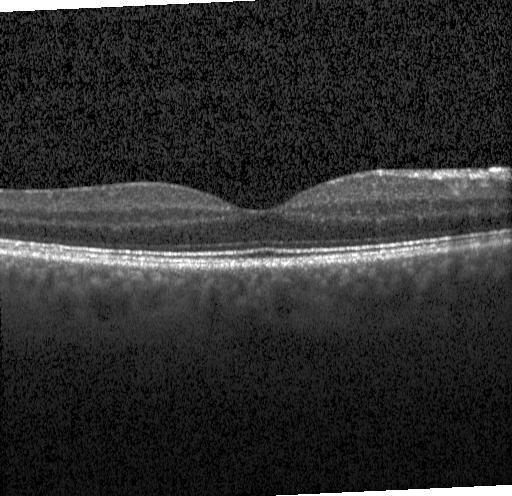 Optical coherence tomography B-scan. Assessment: neither CNV, DME, nor drusen.